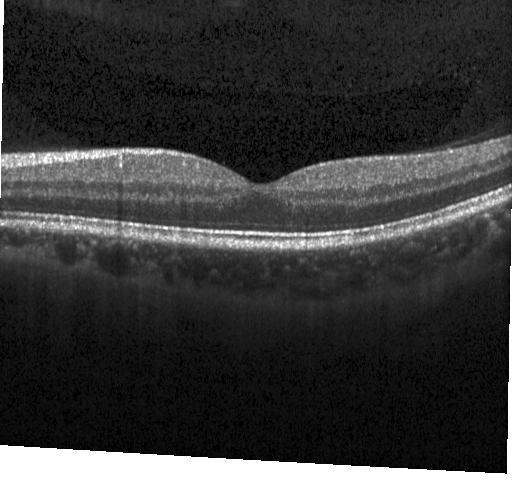 Optical coherence tomography scan, horizontal scan through the fovea, spectral-domain OCT, Heidelberg Spectralis — This B-scan demonstrates no CNV, no DME, and no drusen.